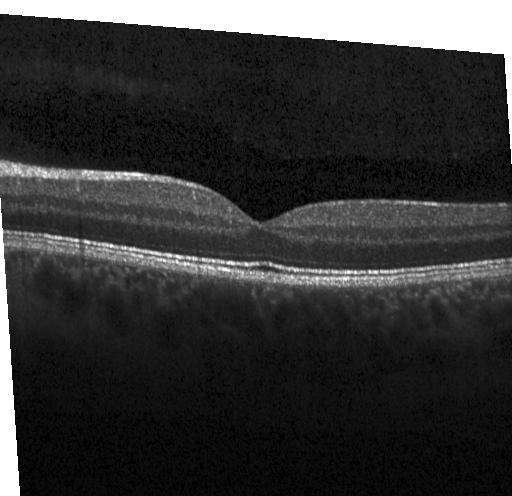 Optical coherence tomography B-scan
No evidence of choroidal neovascularization, diabetic macular edema, or drusen.